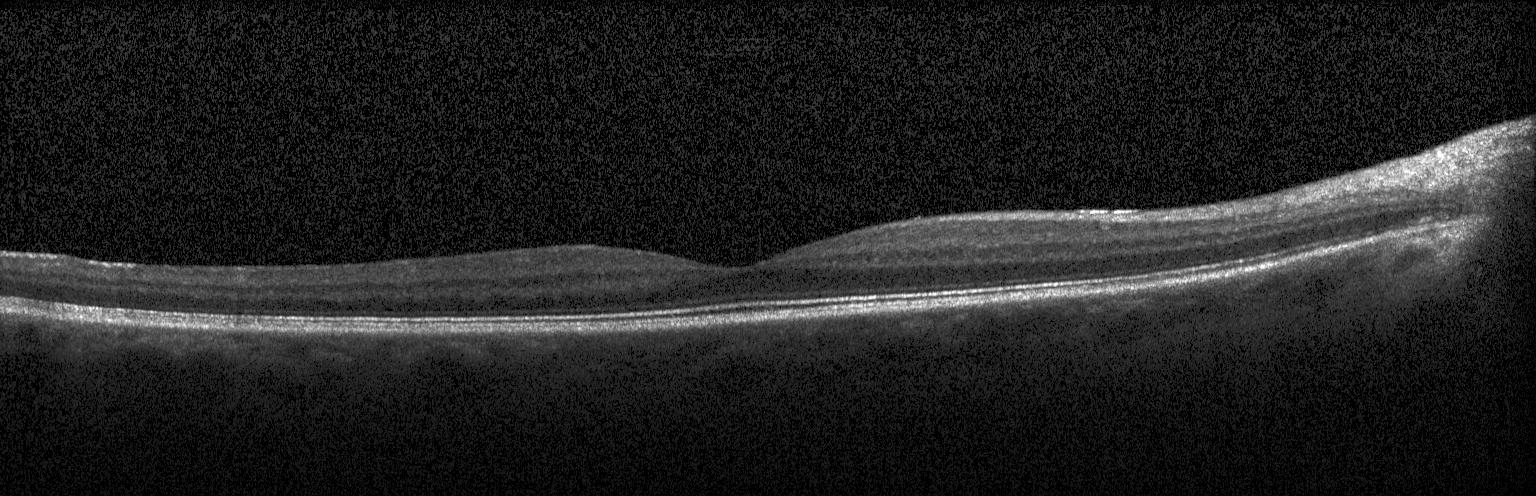
Spectral-domain optical coherence tomography. OCT B-scan. Horizontal scan through the fovea. Heidelberg Spectralis — Impression: no evidence of choroidal neovascularization, diabetic macular edema, or drusen.